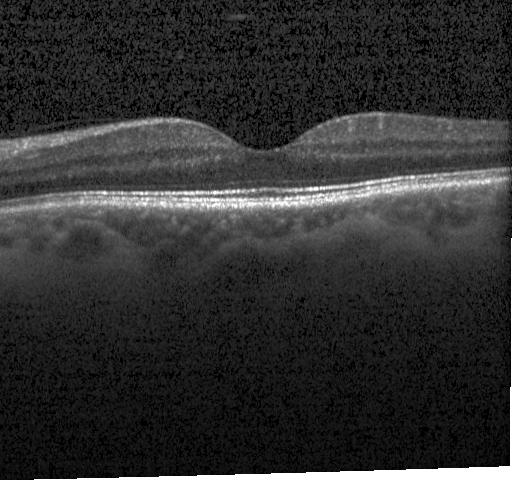
Macular scan; Heidelberg Spectralis OCT system; optical coherence tomography scan. Finding: no choroidal neovascularization, no diabetic macular edema, and no drusen.